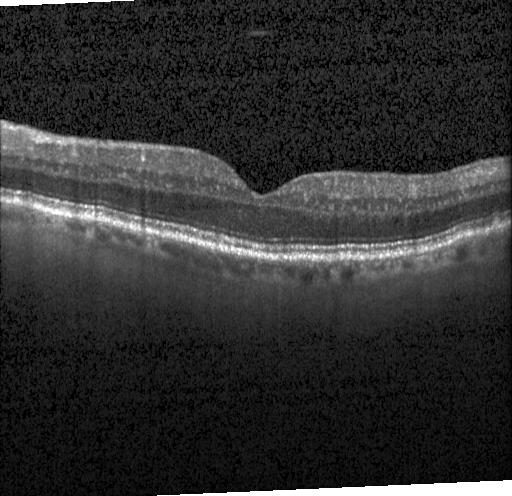

Heidelberg Spectralis. Optical coherence tomography B-scan. Dx: no choroidal neovascularization, no diabetic macular edema, and no drusen.